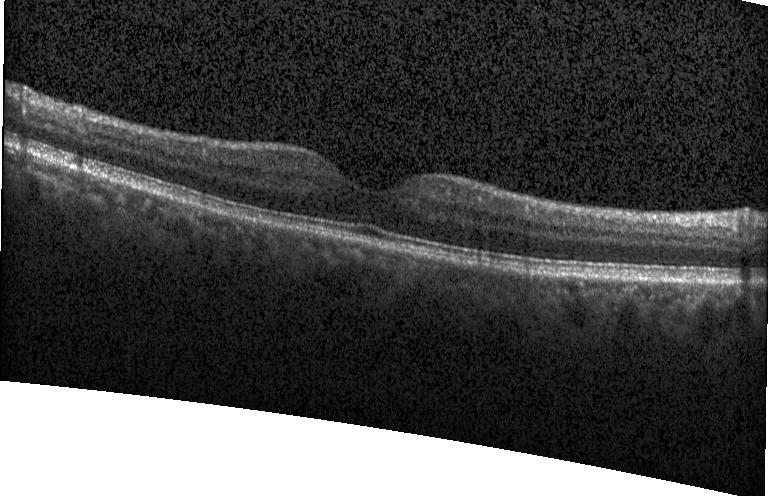 Macular OCT: no choroidal neovascularization, no diabetic macular edema, and no drusen.